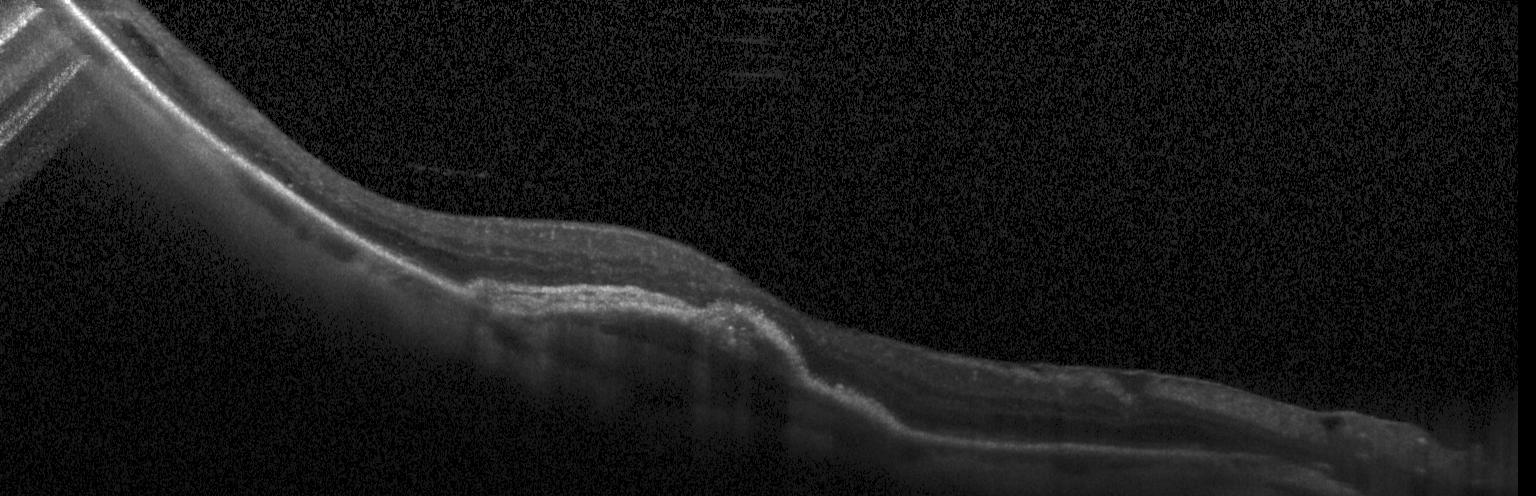 Instrument: Heidelberg Spectralis · fovea-centered · OCT line scan. Assessment: a choroidal neovascular membrane.